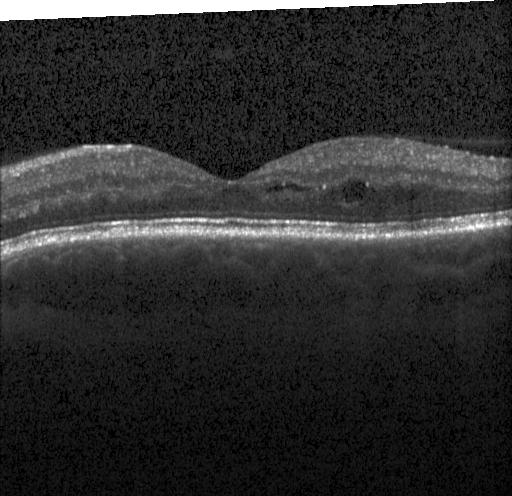

Horizontal scan through the fovea; spectral-domain optical coherence tomography; OCT line scan; Heidelberg Spectralis OCT system — Diagnosis: diabetic macular edema (DME).